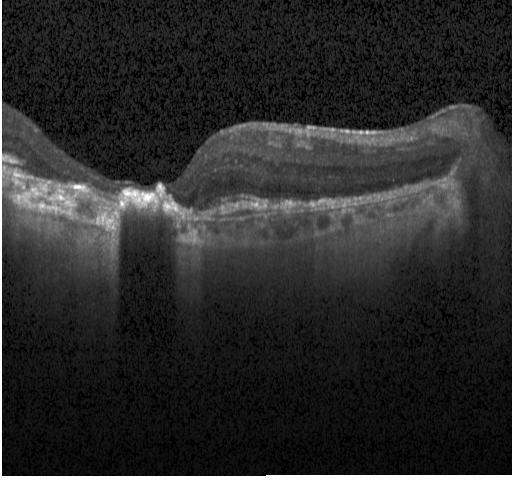 SD-OCT. Centered on the fovea. Heidelberg Spectralis. Optical coherence tomography B-scan. Assessment: choroidal neovascularization.